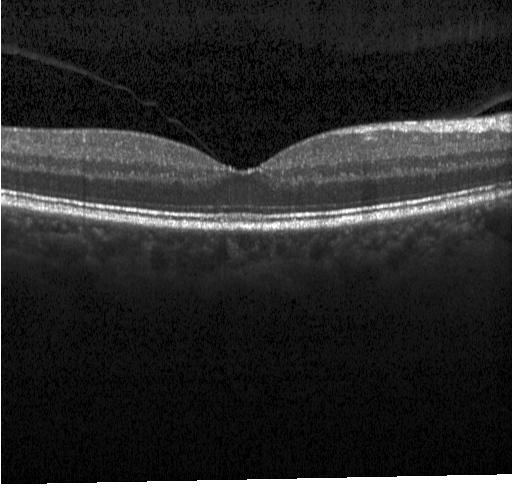

Heidelberg Spectralis. Retinal OCT cross-section. The scan shows no choroidal neovascularization, no diabetic macular edema, and no drusen.